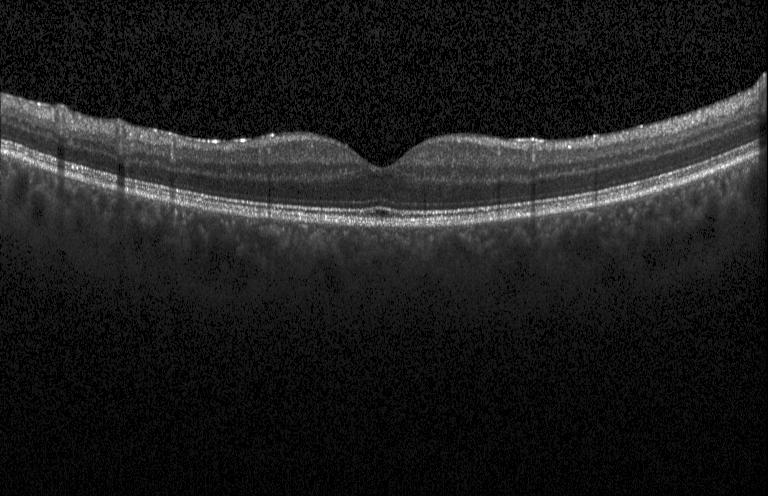
Retinal OCT cross-section. Finding: no evidence of choroidal neovascularization, diabetic macular edema, or drusen.